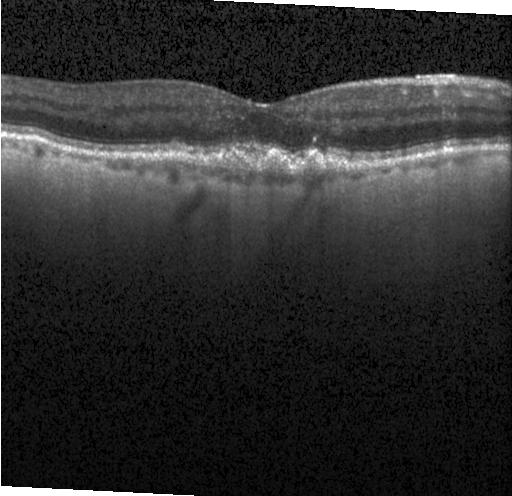 Impression: sub-RPE drusenoid deposits.